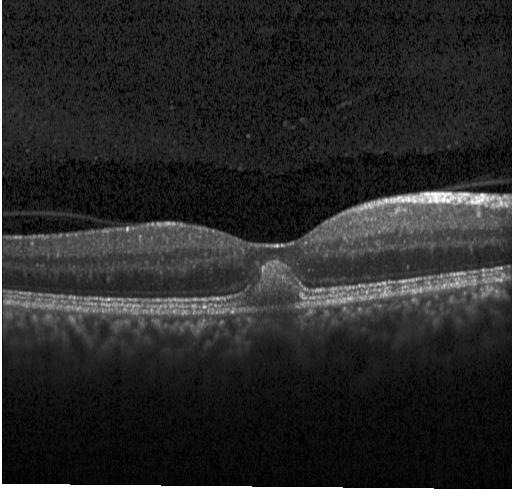

Optical coherence tomography B-scan, spectral-domain OCT, macular scan. Finding: choroidal neovascularization.